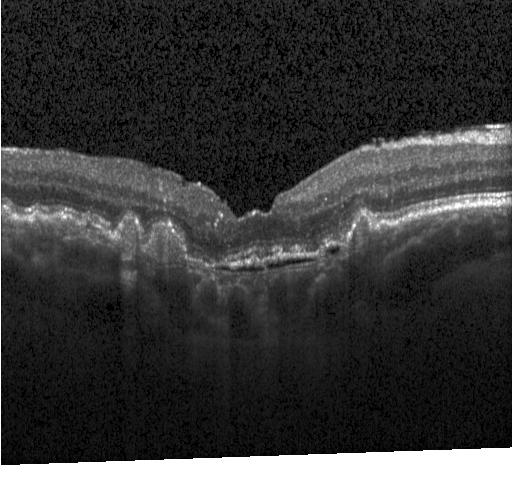 SD-OCT; retinal OCT cross-section. Impression: a choroidal neovascular membrane.